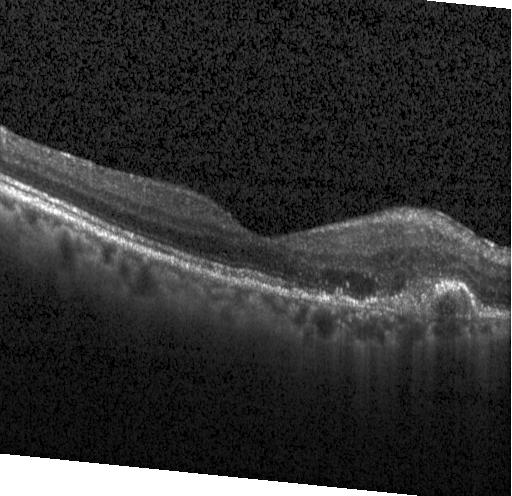

Spectral-domain optical coherence tomography; retinal OCT B-scan; acquired on a Heidelberg Spectralis; macular scan — Choroidal neovascularization (CNV).